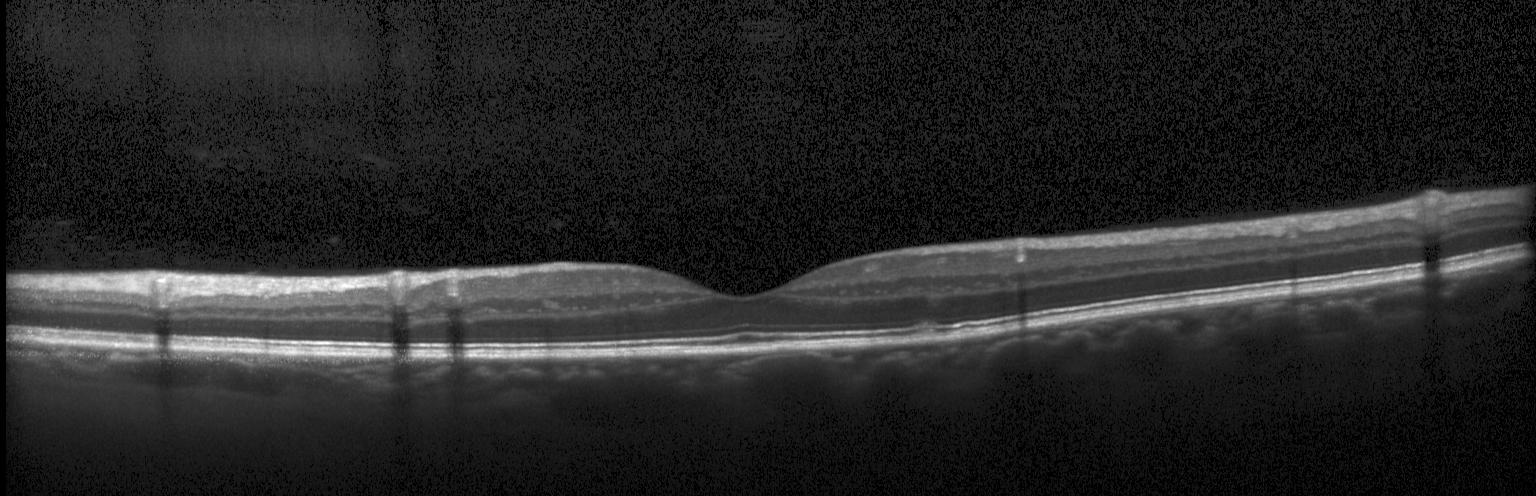
Diagnosis: no choroidal neovascularization, diabetic macular edema, or drusen.